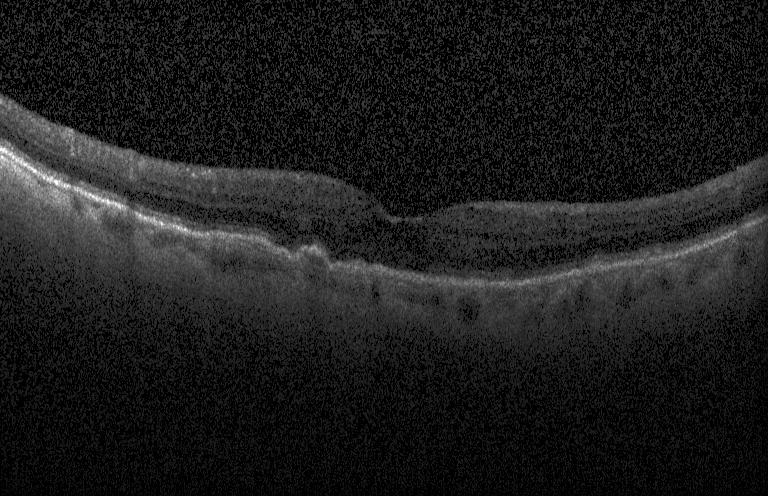

Finding: a choroidal neovascular membrane.